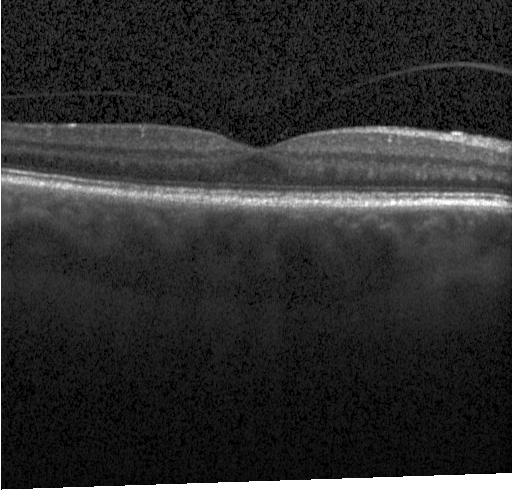 OCT B-scan showing no choroidal neovascularization, no diabetic macular edema, and no drusen.